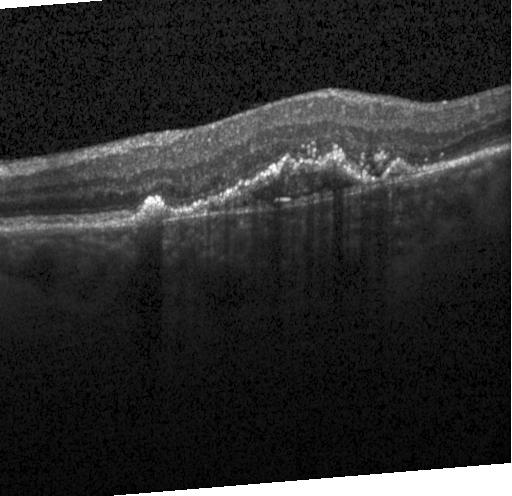

Spectral-domain OCT, retinal OCT cross-section — Dx: choroidal neovascularization (CNV).